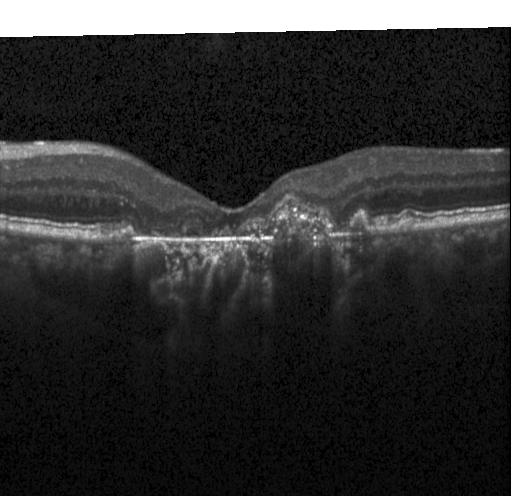

Optical coherence tomography scan. Spectral-domain optical coherence tomography — Impression: a choroidal neovascular membrane.